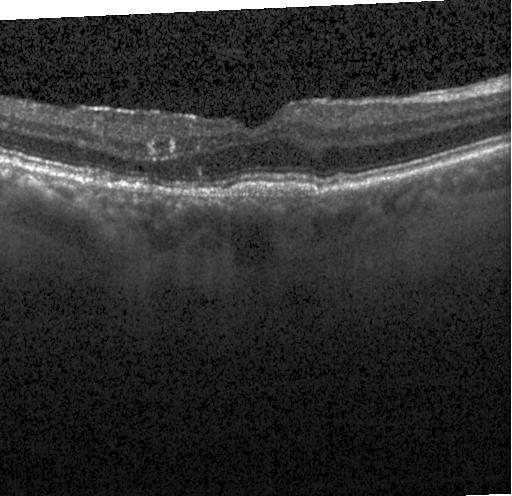
Optical coherence tomography scan. Spectral-domain OCT. Impression: CNV.